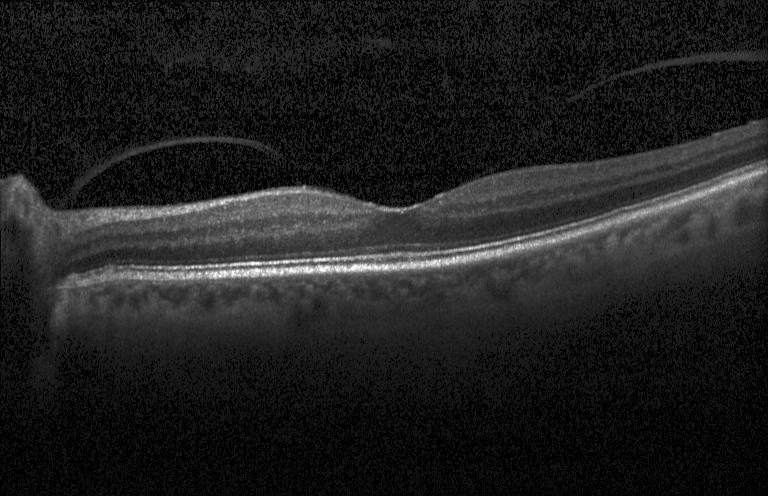

Optical coherence tomography scan. Heidelberg Spectralis. Through the macula. SD-OCT
This B-scan demonstrates no evidence of CNV, DME, or drusen.